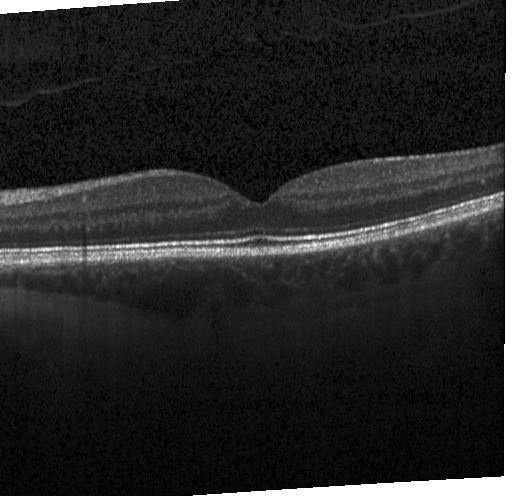
Retinal OCT cross-section, spectral-domain OCT, Heidelberg Spectralis — Dx: no choroidal neovascularization, no diabetic macular edema, and no drusen.